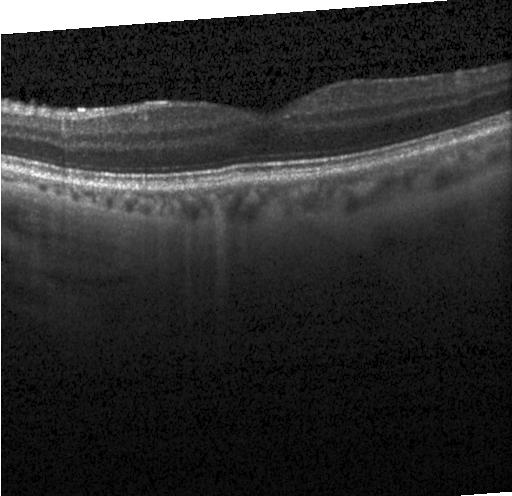
Retinal OCT B-scan. Through the macula. Heidelberg Spectralis OCT system. Spectral-domain OCT. No evidence of choroidal neovascularization, diabetic macular edema, or drusen.